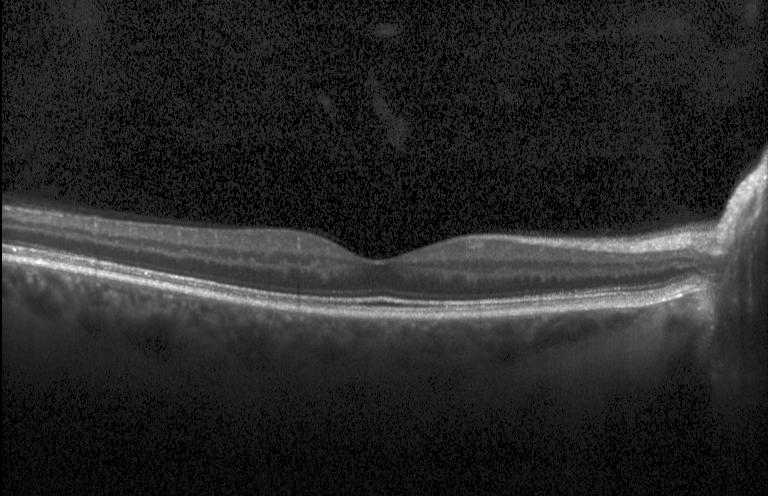
OCT B-scan — Impression: no evidence of CNV, DME, or drusen.